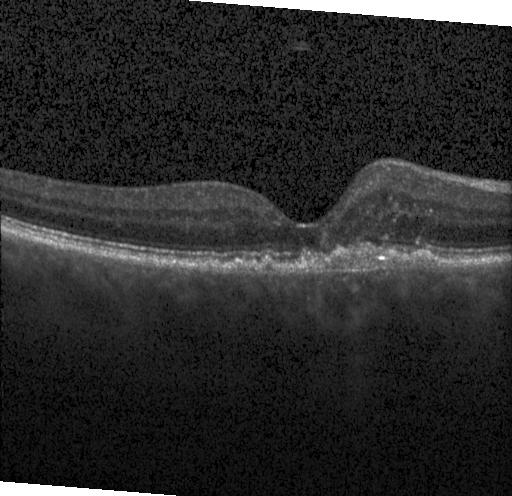 Impression: CNV.